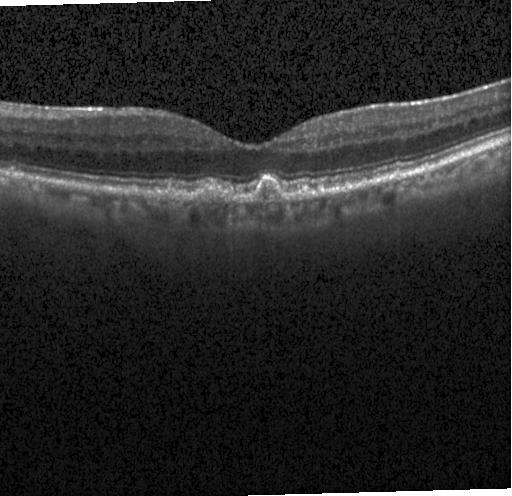

Drusen.